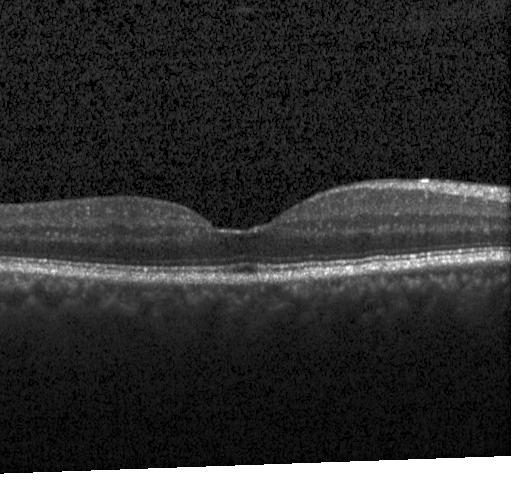
Through the macula · spectral-domain OCT · instrument: Heidelberg Spectralis · optical coherence tomography B-scan. Diagnosis: no CNV, no DME, and no drusen.